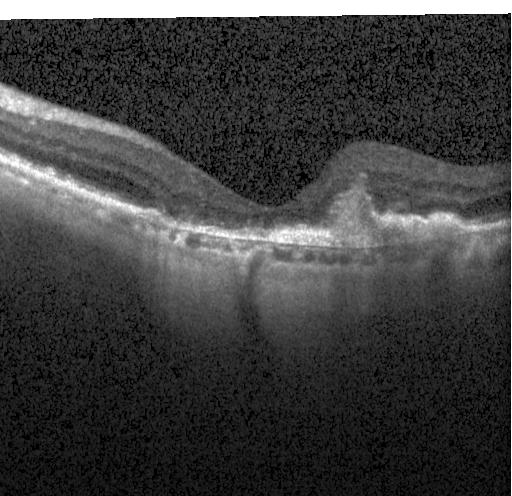 Optical coherence tomography scan; horizontal scan through the fovea; SD-OCT
Macular OCT: CNV.